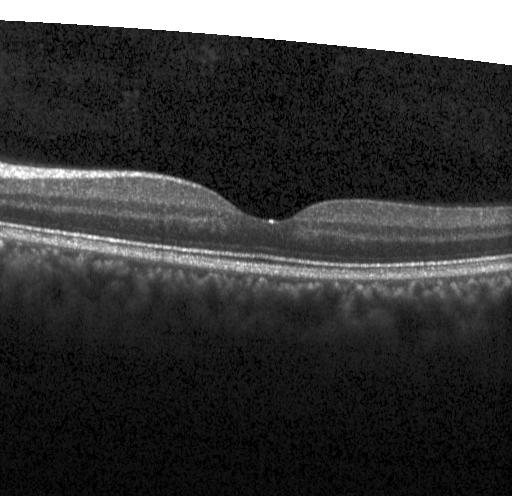
Through the macula. Optical coherence tomography scan. Instrument: Heidelberg Spectralis. Spectral-domain OCT — Diagnosis: no evidence of choroidal neovascularization, diabetic macular edema, or drusen.